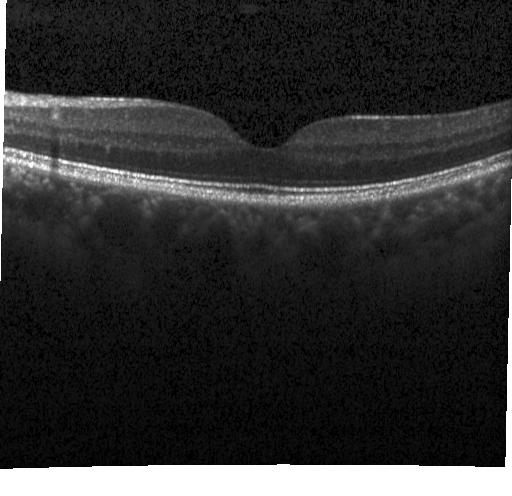

SD-OCT · retinal OCT B-scan — Impression: no choroidal neovascularization, no diabetic macular edema, and no drusen.